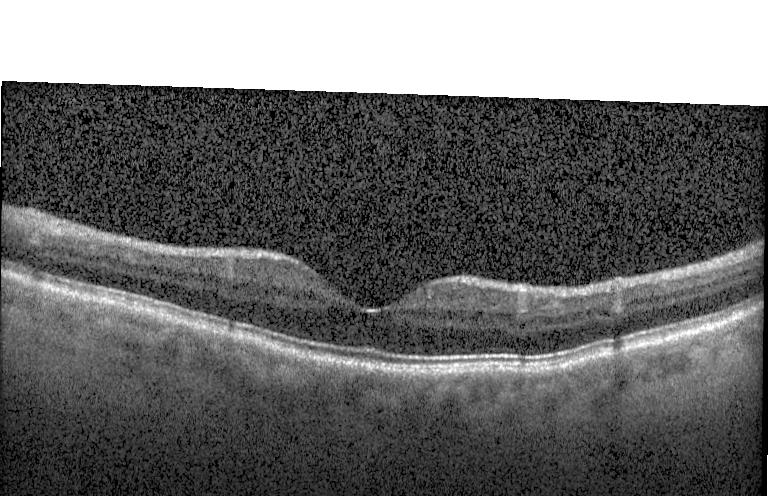

Instrument: Heidelberg Spectralis, SD-OCT, optical coherence tomography scan.
Dx: neither CNV, DME, nor drusen.